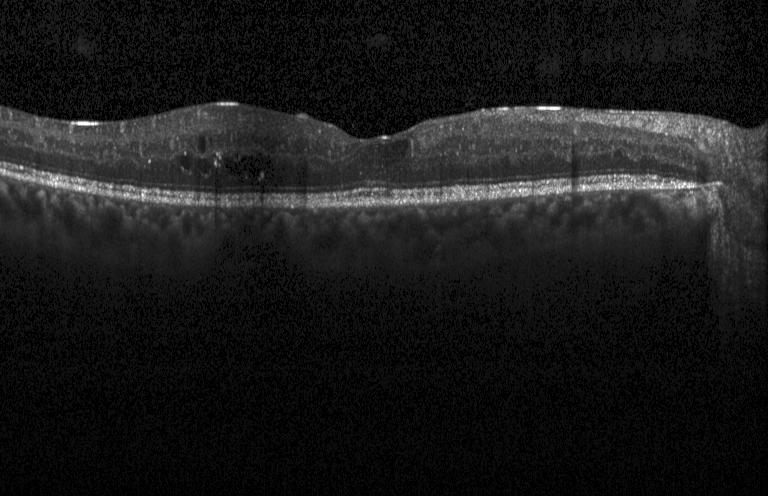 Through the macula; OCT line scan; Heidelberg Spectralis OCT system; SD-OCT — OCT finding: diabetic macular edema (DME).